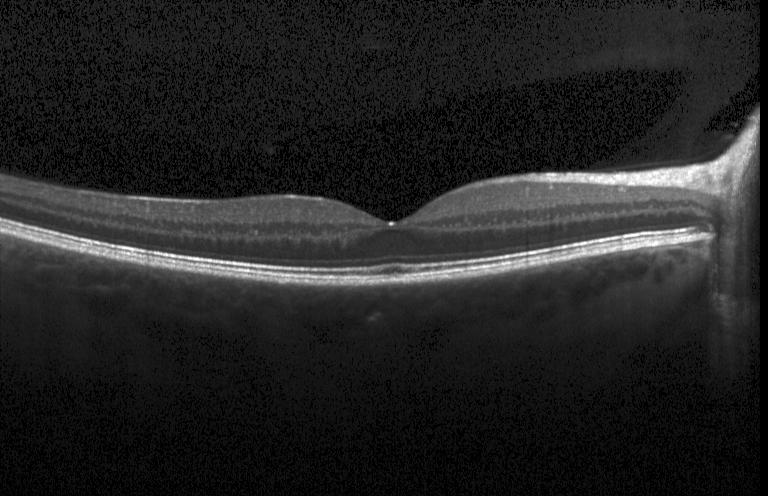 Macular OCT demonstrating no choroidal neovascularization, no diabetic macular edema, and no drusen.